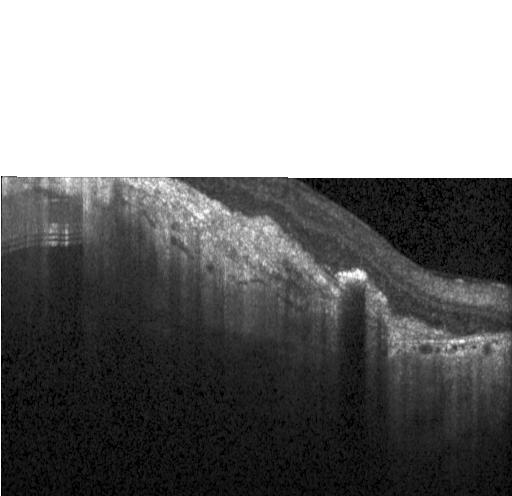 SD-OCT. OCT B-scan — A choroidal neovascular membrane.